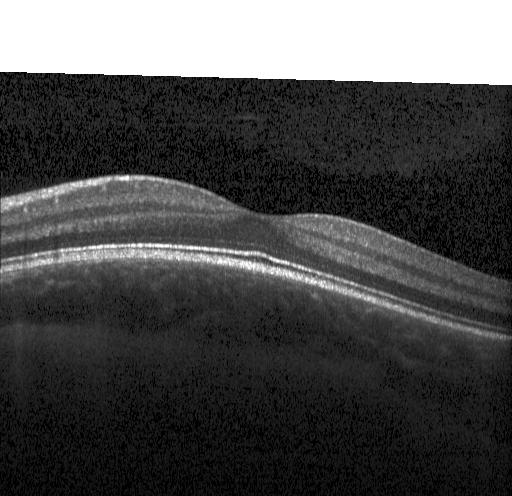

Optical coherence tomography B-scan
This B-scan demonstrates no evidence of CNV, DME, or drusen.